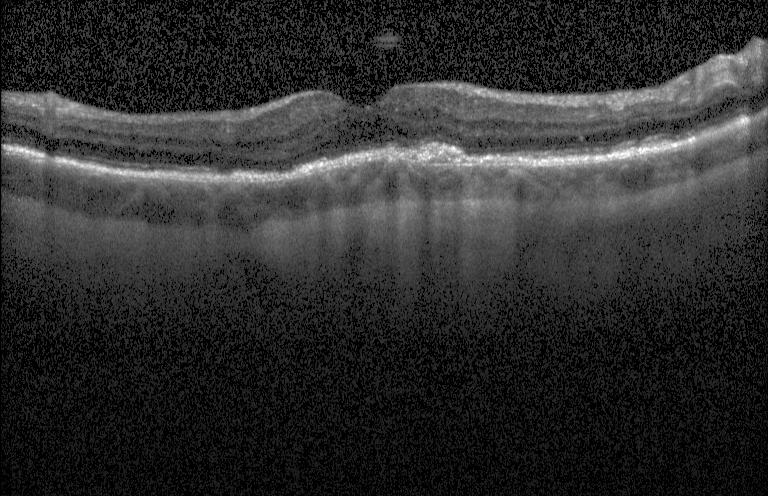
Macular OCT: choroidal neovascularization.